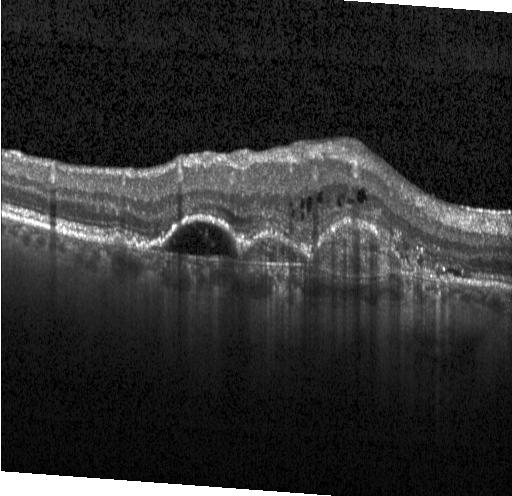 Optical coherence tomography B-scan · SD-OCT
Diagnosis: choroidal neovascularization (CNV).